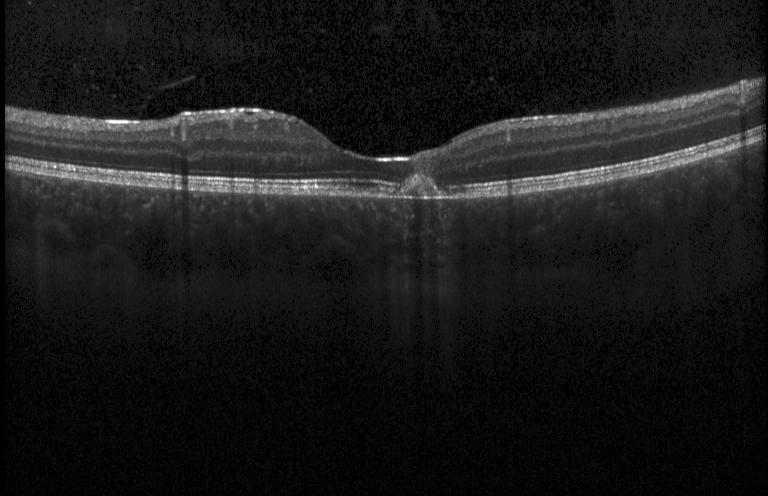

Assessment: a choroidal neovascular membrane.